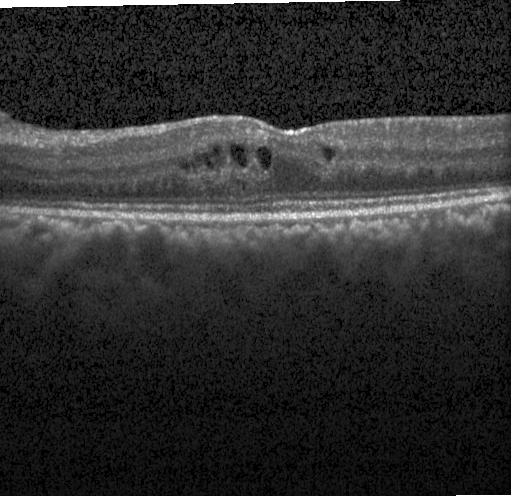 Optical coherence tomography scan, centered on the fovea, spectral-domain OCT
Macular OCT: DME.